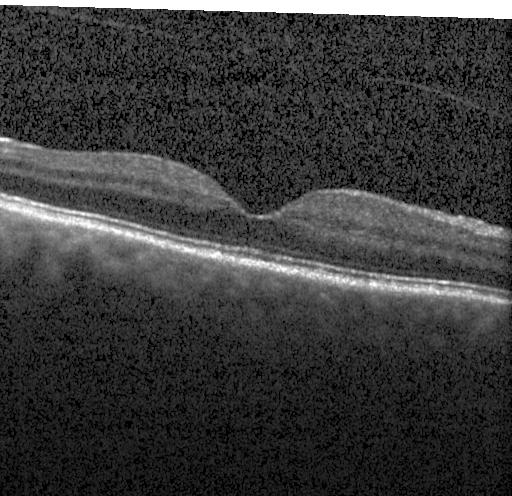 Macular OCT: no choroidal neovascularization, no diabetic macular edema, and no drusen.